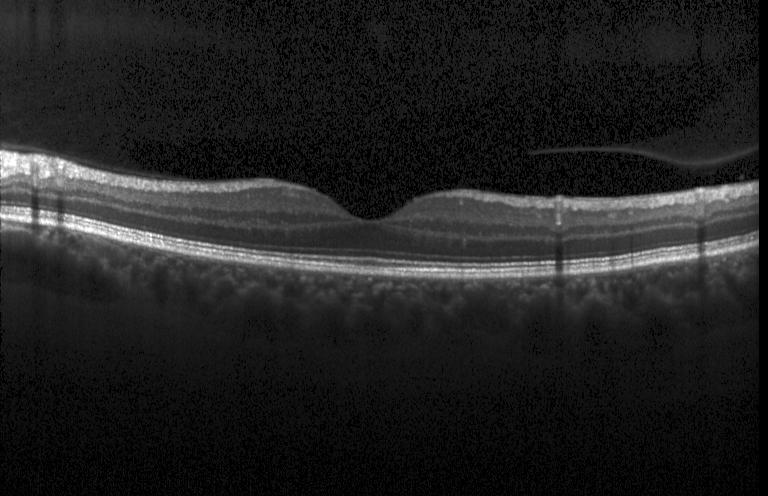
The scan shows no CNV, no DME, and no drusen.